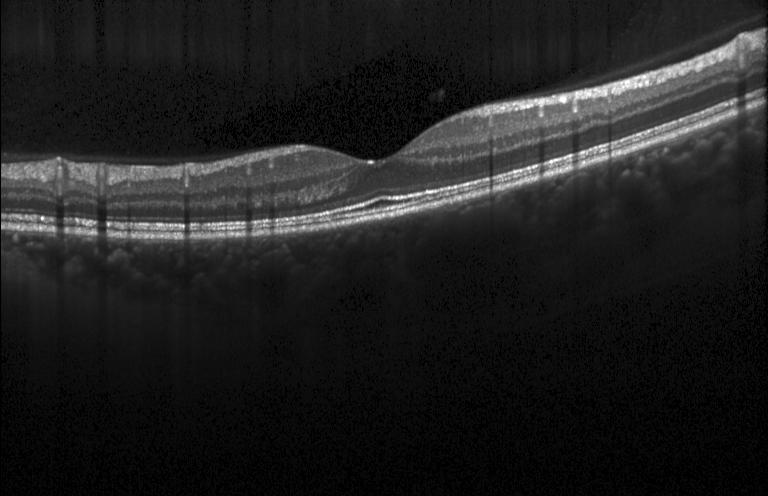
Optical coherence tomography scan — Impression: no choroidal neovascularization, diabetic macular edema, or drusen.